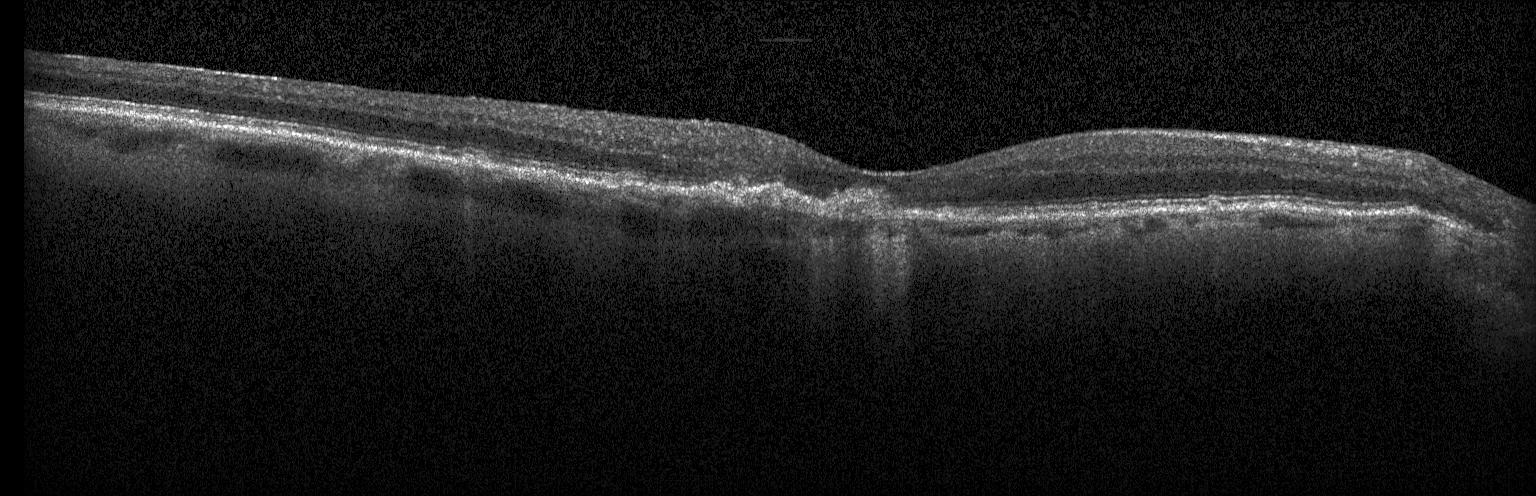 Impression: a choroidal neovascular membrane.